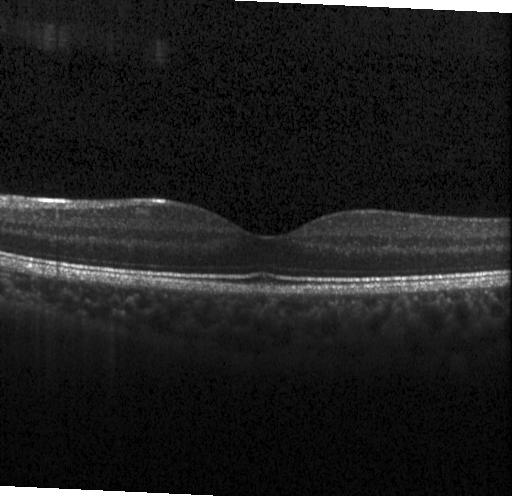 Assessment: neither choroidal neovascularization, diabetic macular edema, nor drusen.